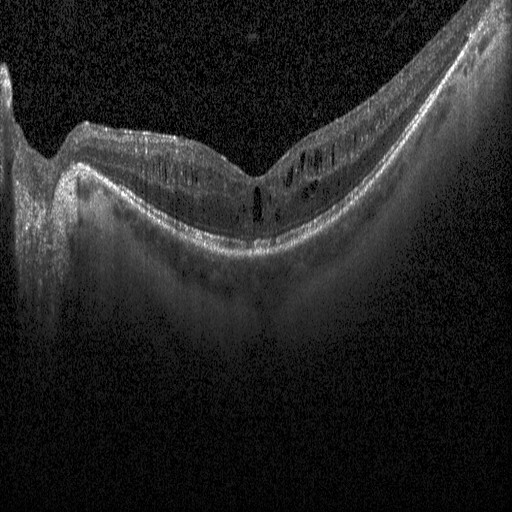
This B-scan demonstrates diabetic macular edema.